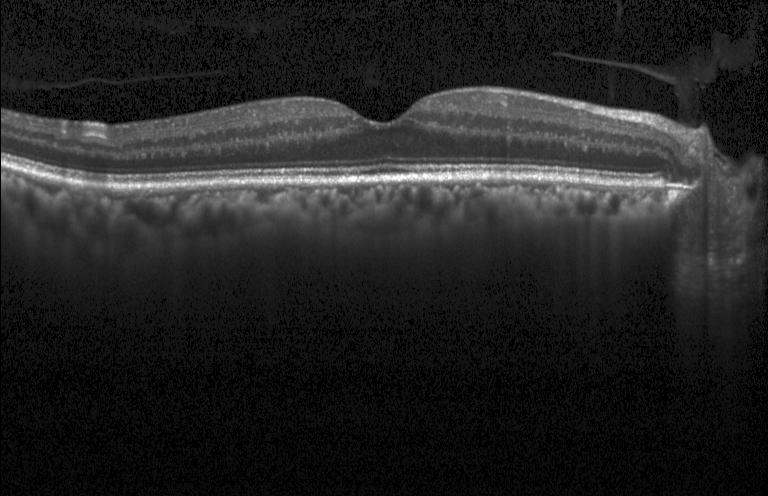 Optical coherence tomography B-scan, through the macula. Neither choroidal neovascularization, diabetic macular edema, nor drusen.